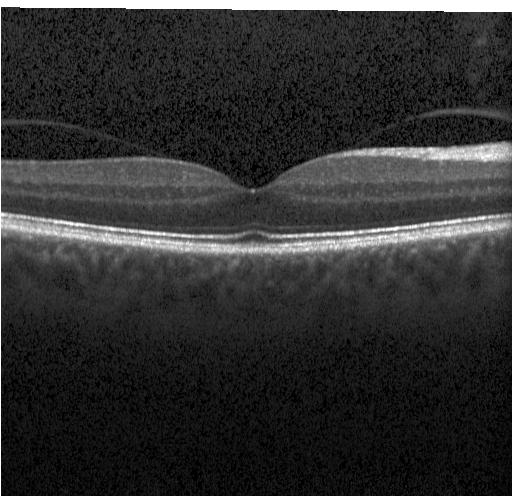

OCT line scan.
Finding: no evidence of choroidal neovascularization, diabetic macular edema, or drusen.